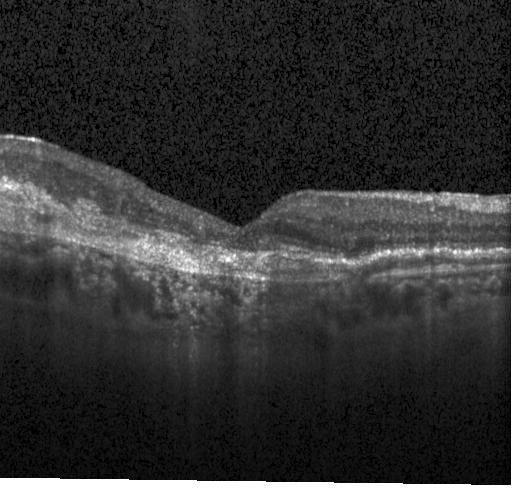 Instrument: Heidelberg Spectralis; SD-OCT; optical coherence tomography scan — CNV.